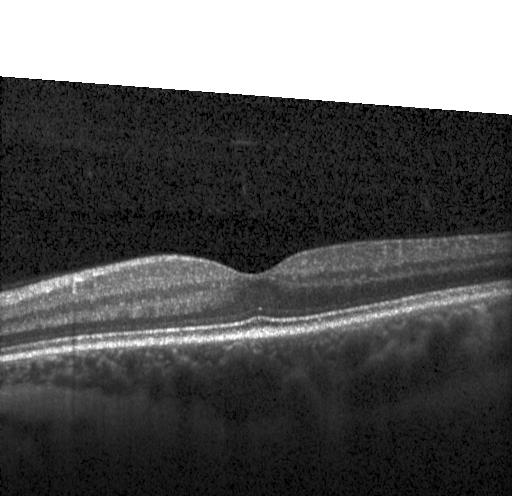 Heidelberg Spectralis · retinal OCT B-scan · SD-OCT · centered on the fovea — Dx: neither choroidal neovascularization, diabetic macular edema, nor drusen.